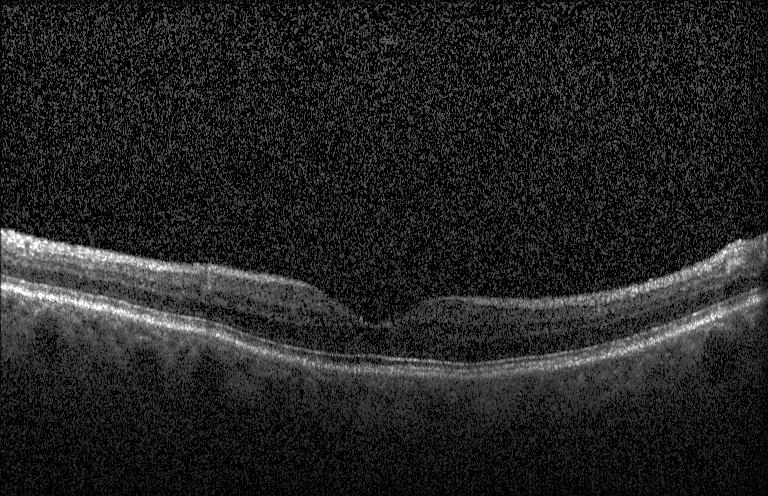

OCT B-scan — Impression: no choroidal neovascularization, no diabetic macular edema, and no drusen.